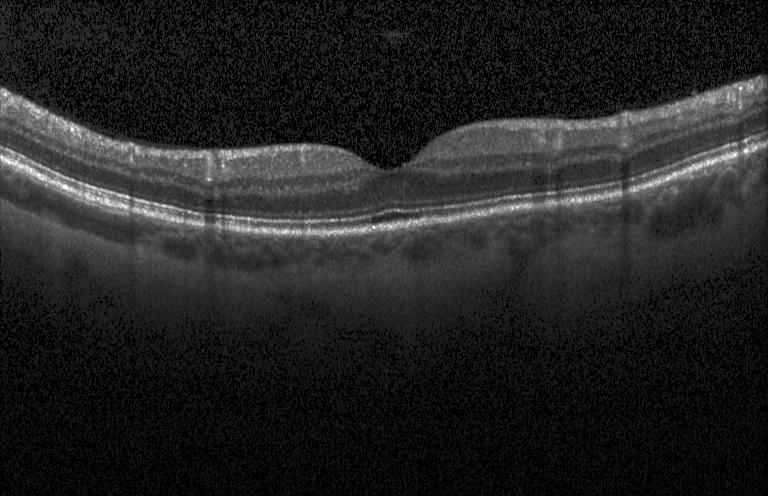
Instrument: Heidelberg Spectralis, fovea-centered, OCT line scan, SD-OCT.
This B-scan demonstrates no choroidal neovascularization, diabetic macular edema, or drusen.